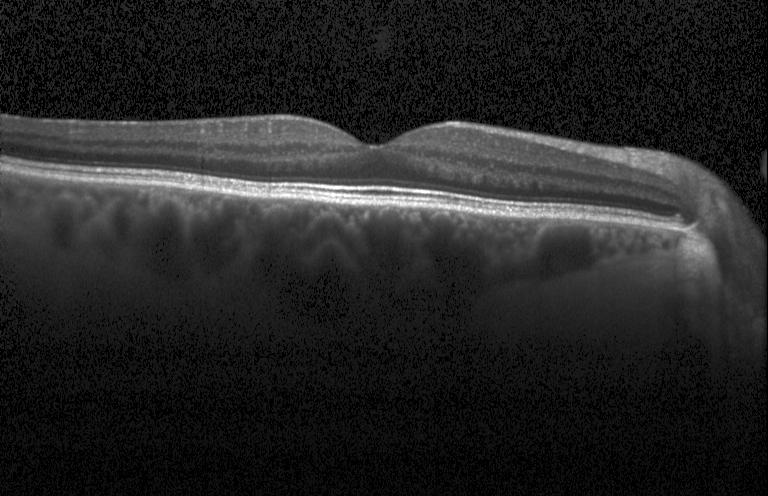

Retinal OCT cross-section. Instrument: Heidelberg Spectralis. Horizontal scan through the fovea. Spectral-domain optical coherence tomography
Macular OCT: no CNV, DME, or drusen.